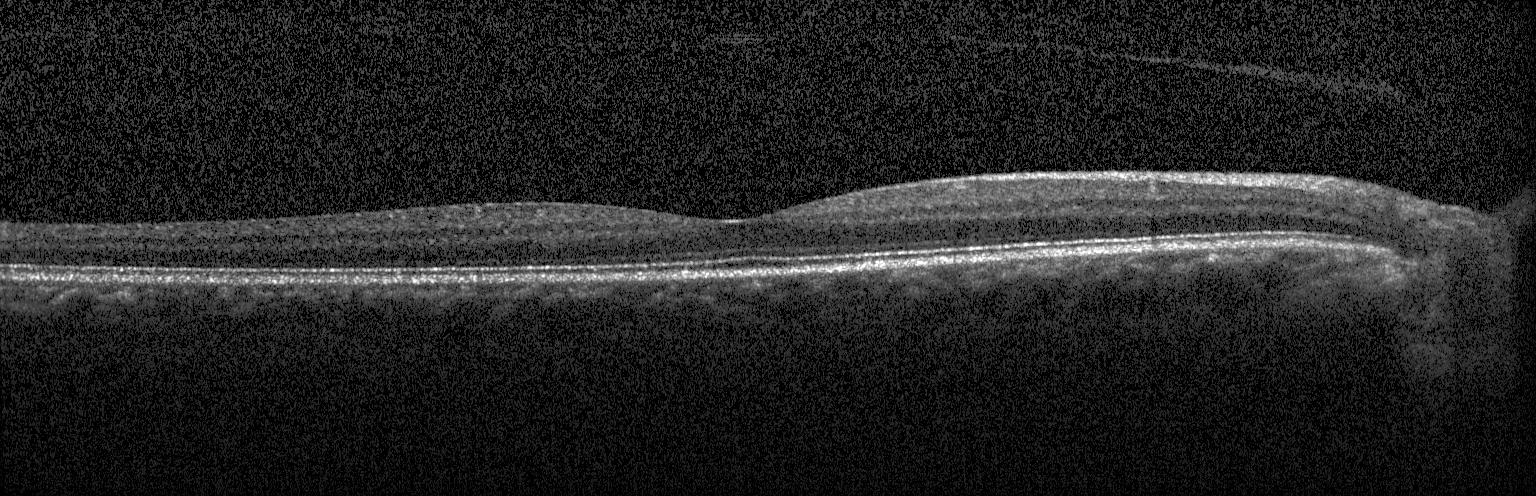
No choroidal neovascularization, diabetic macular edema, or drusen.